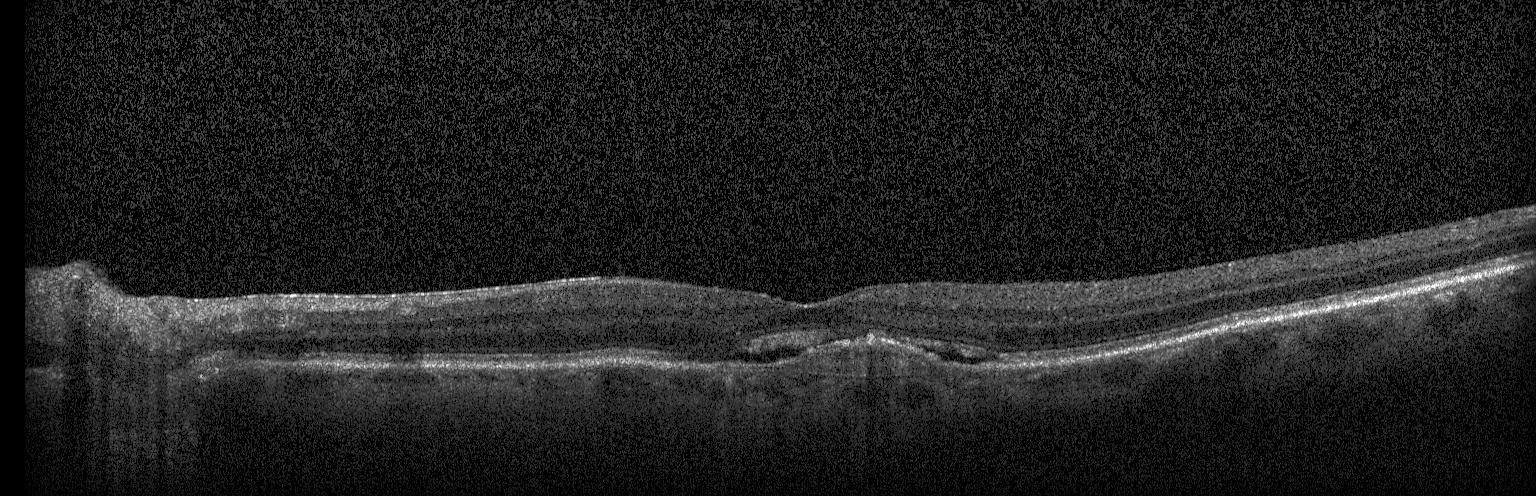
Retinal OCT B-scan · spectral-domain OCT. Diagnosis: CNV.